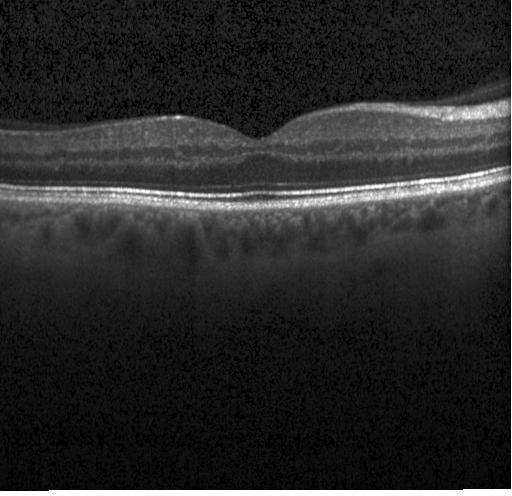
Diagnosis: no evidence of choroidal neovascularization, diabetic macular edema, or drusen.